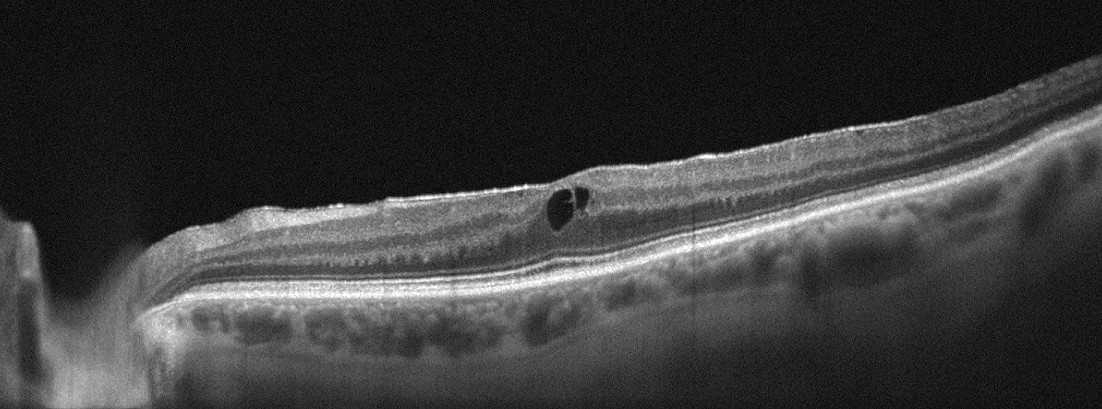 Instrument: Optovue Avanti RTVue XR · fovea-centered · OCT B-scan. Finding: epiretinal membrane.